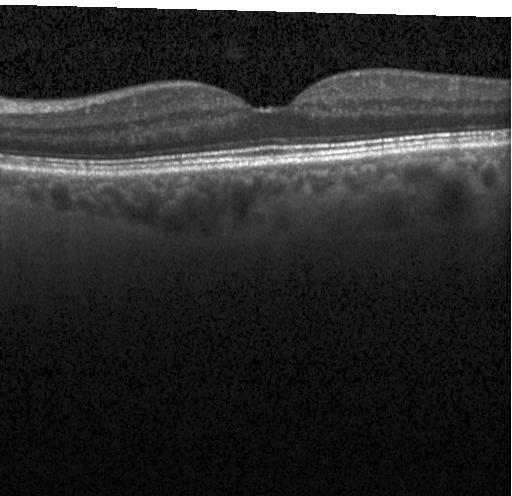 Fovea-centered, OCT line scan — Dx: no evidence of choroidal neovascularization, diabetic macular edema, or drusen.